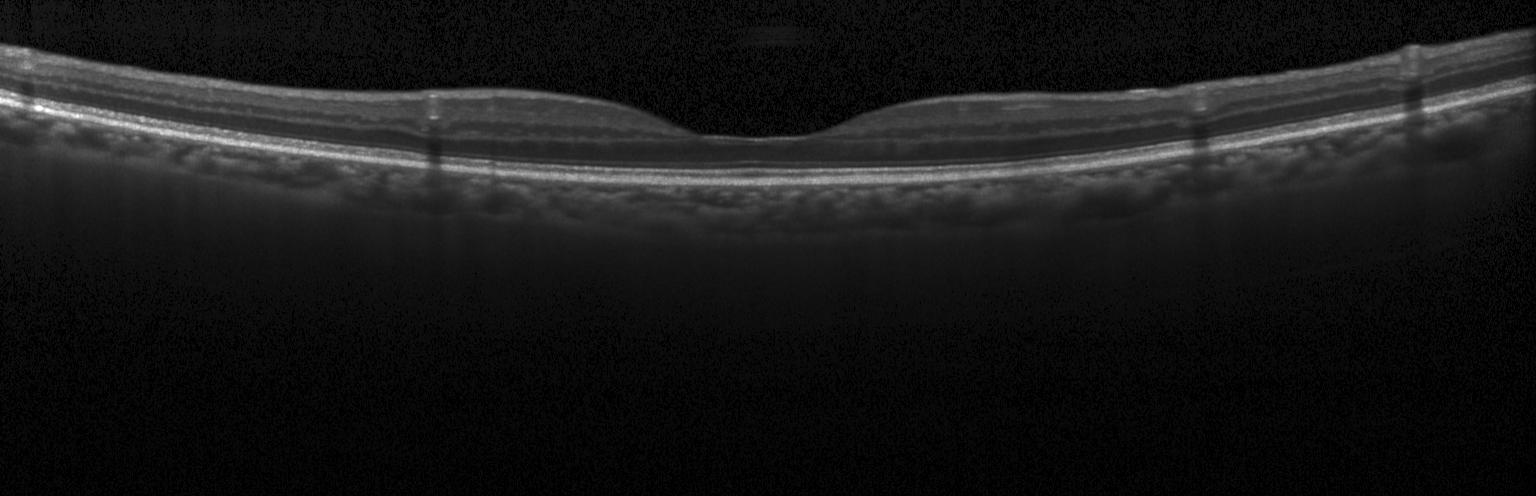

OCT B-scan, centered on the fovea — Macular OCT: no CNV, no DME, and no drusen.